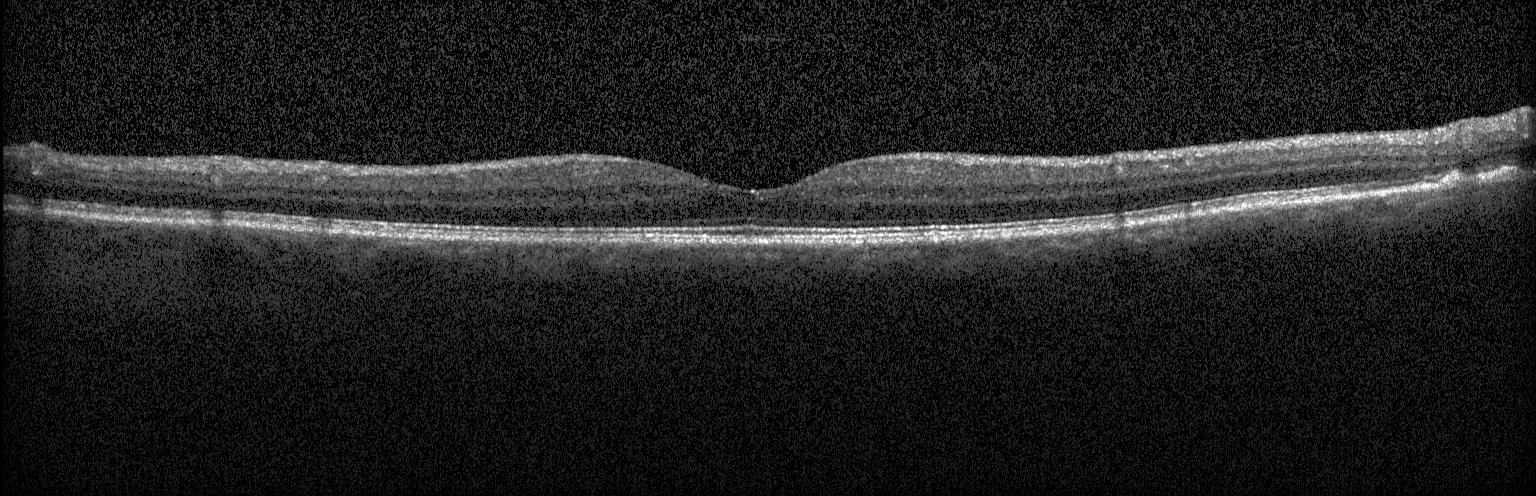

Retinal OCT B-scan.
No evidence of choroidal neovascularization, diabetic macular edema, or drusen.